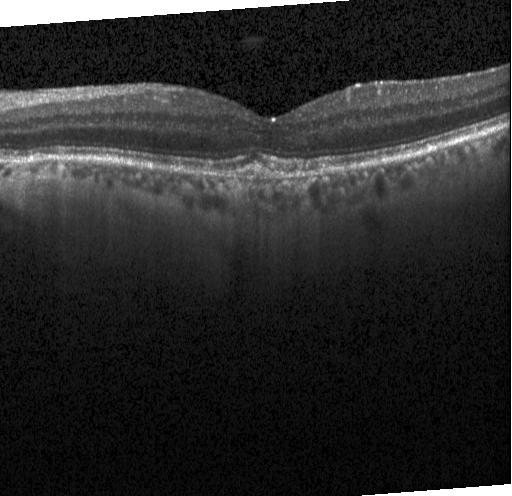

Macular OCT demonstrating a choroidal neovascular membrane.